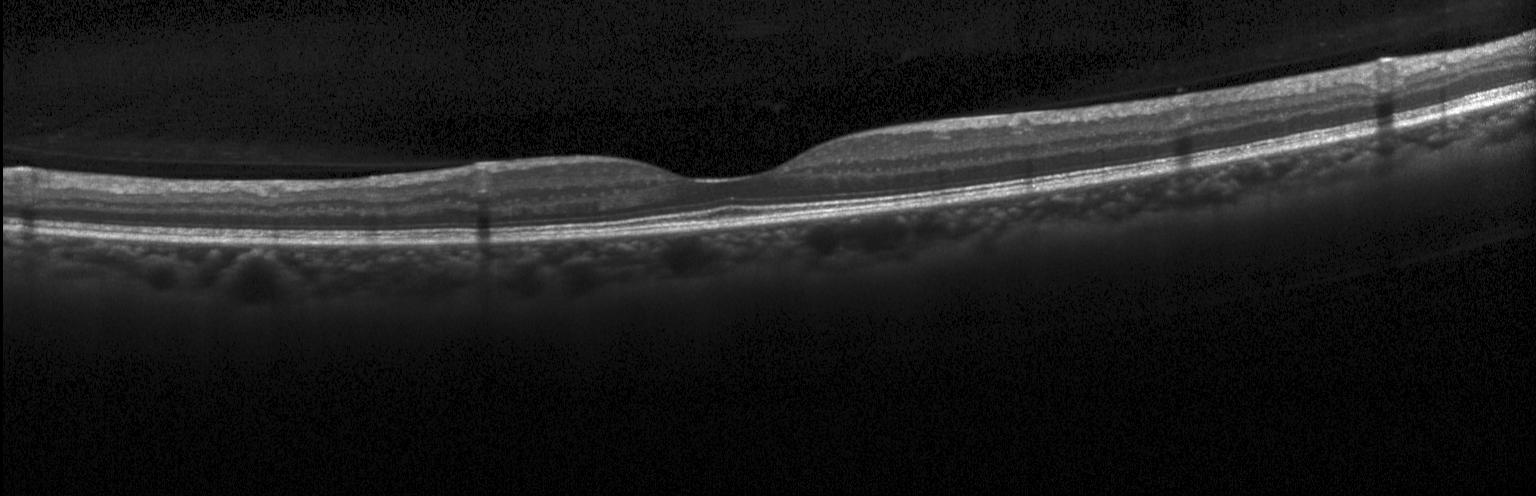

Diagnosis: no choroidal neovascularization, no diabetic macular edema, and no drusen.